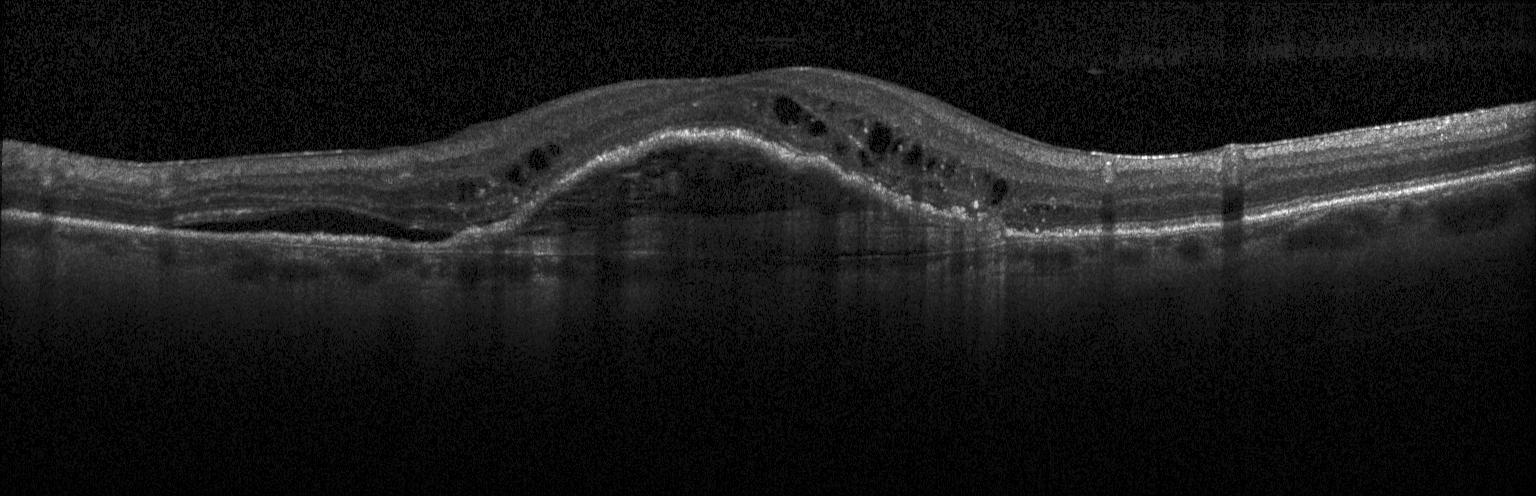 SD-OCT. Instrument: Heidelberg Spectralis. Optical coherence tomography B-scan
OCT finding: CNV.